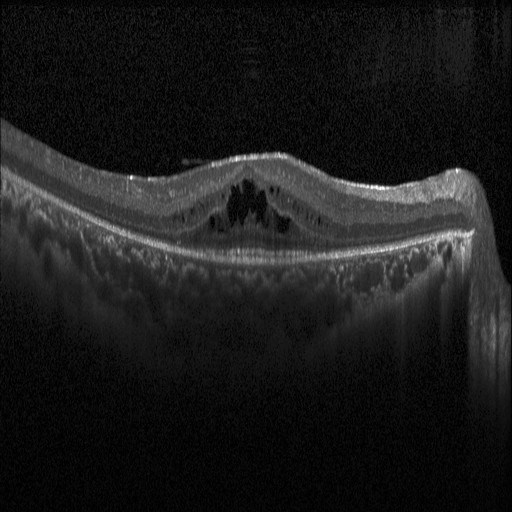 Impression: diabetic macular edema.